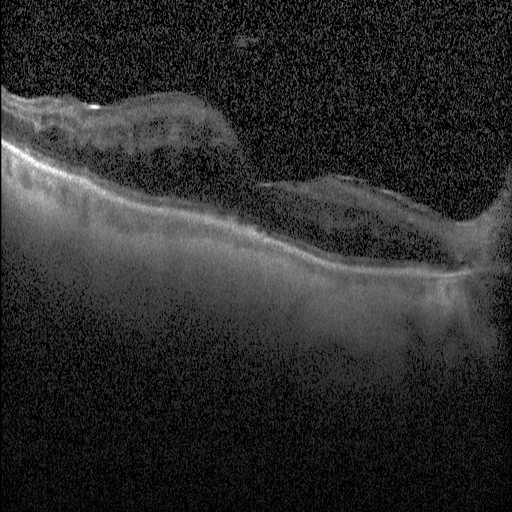

Assessment: diabetic macular edema.